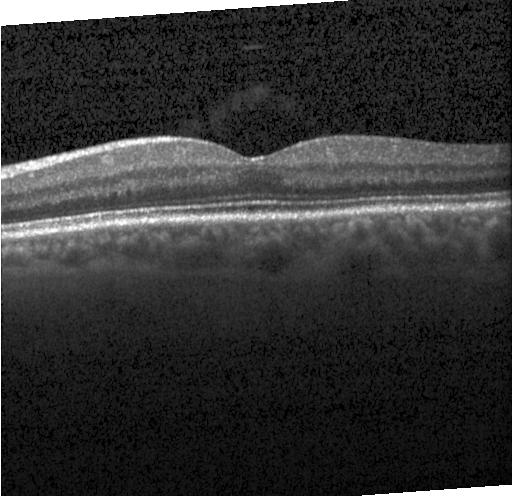

Retinal OCT cross-section showing neither CNV, DME, nor drusen.